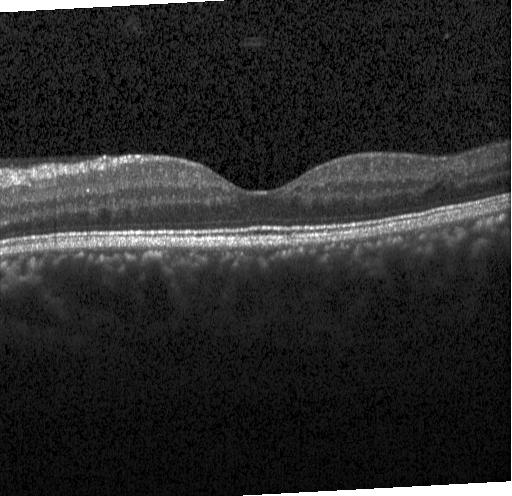

Retinal OCT B-scan
Diagnosis: no CNV, DME, or drusen.